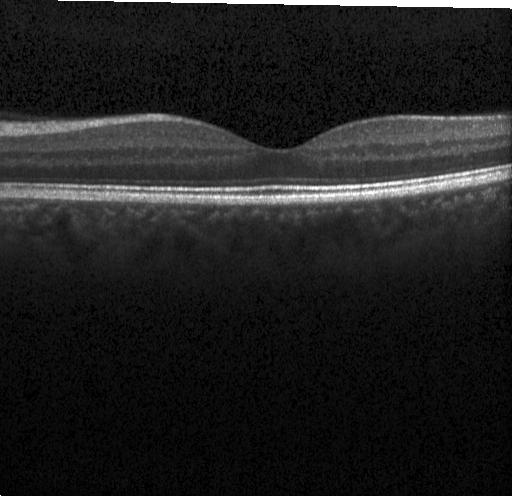
Centered on the fovea · optical coherence tomography scan. Impression: no CNV, no DME, and no drusen.